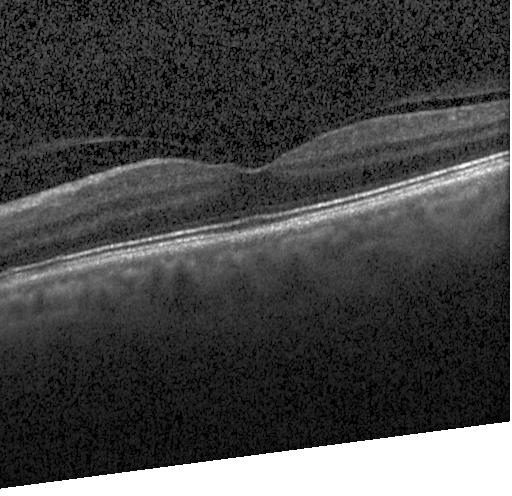
Instrument: Heidelberg Spectralis; retinal OCT B-scan; horizontal scan through the fovea; spectral-domain optical coherence tomography.
This B-scan demonstrates no CNV, no DME, and no drusen.